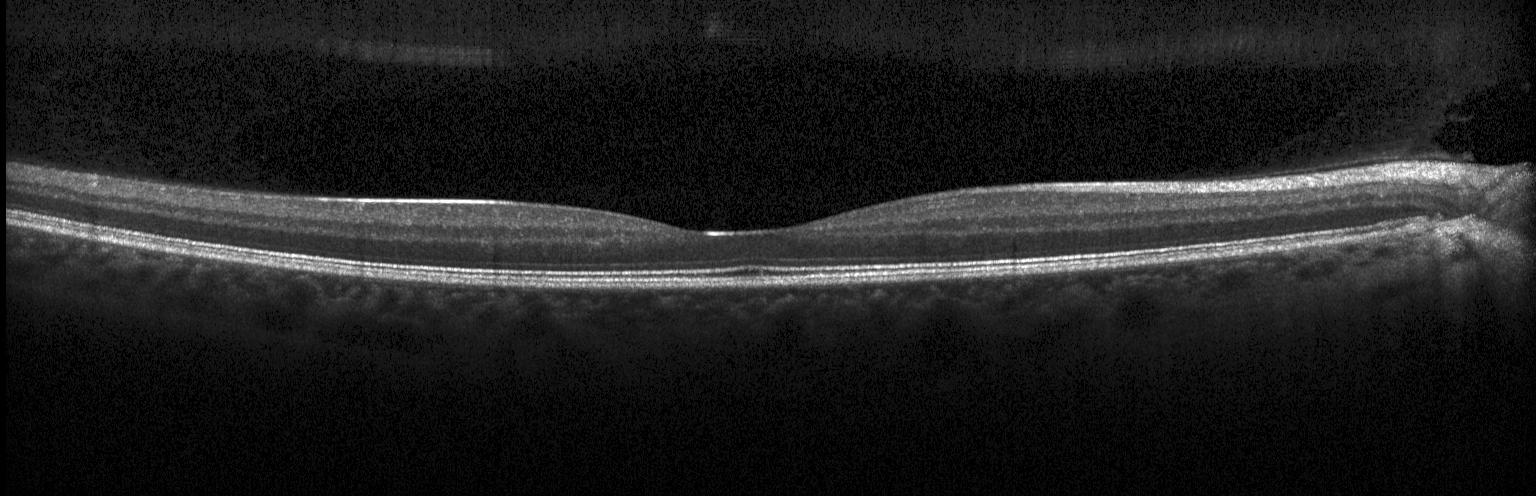

Optical coherence tomography scan.
OCT finding: no choroidal neovascularization, no diabetic macular edema, and no drusen.